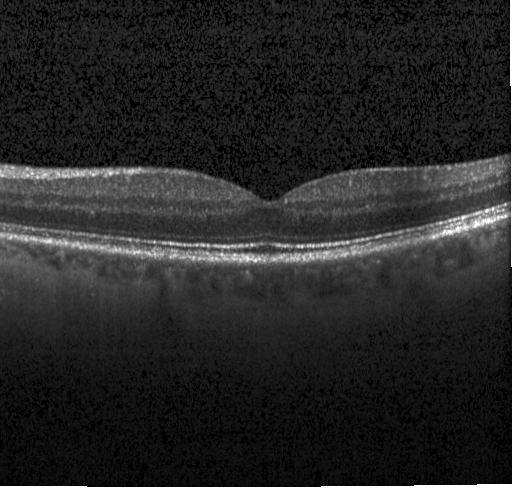
Instrument: Heidelberg Spectralis, optical coherence tomography B-scan, SD-OCT — OCT finding: no choroidal neovascularization, no diabetic macular edema, and no drusen.